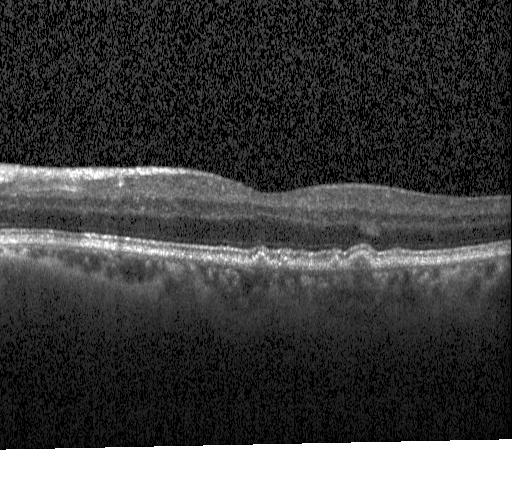

Spectral-domain OCT B-scan: sub-RPE drusenoid deposits.